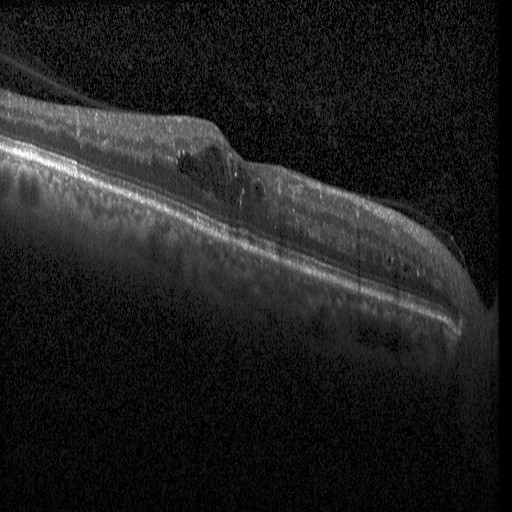
Spectral-domain OCT, optical coherence tomography B-scan, instrument: Heidelberg Spectralis.
Diagnosis: DME.